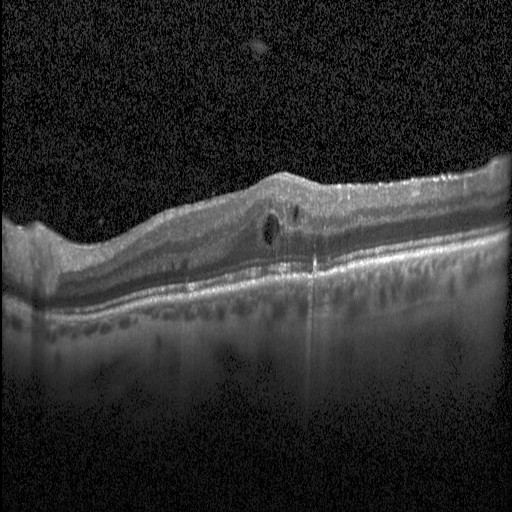 Spectral-domain optical coherence tomography. OCT B-scan. Through the macula. Impression: diabetic macular edema (DME).